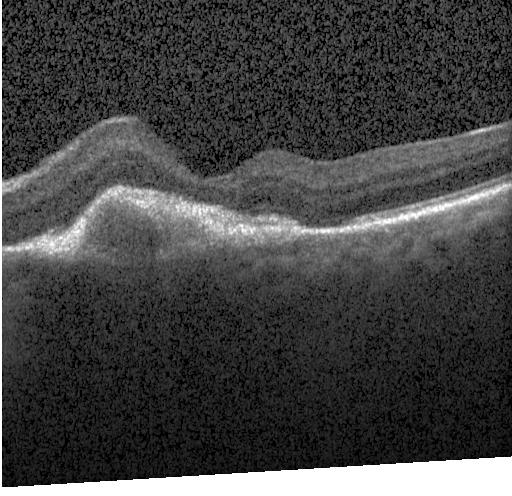

OCT finding: choroidal neovascularization.